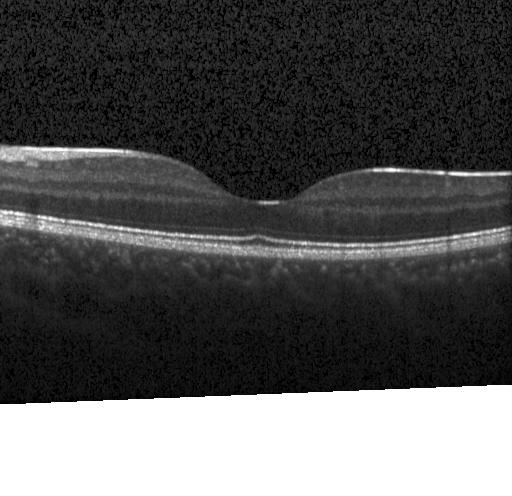

OCT B-scan; spectral-domain optical coherence tomography — Diagnosis: no choroidal neovascularization, no diabetic macular edema, and no drusen.